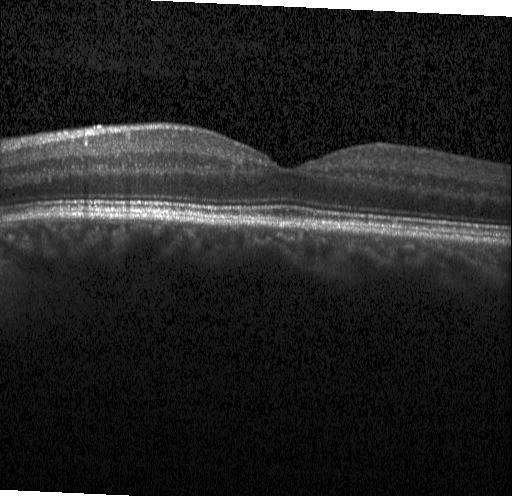

Centered on the fovea · retinal OCT cross-section. No choroidal neovascularization, diabetic macular edema, or drusen.